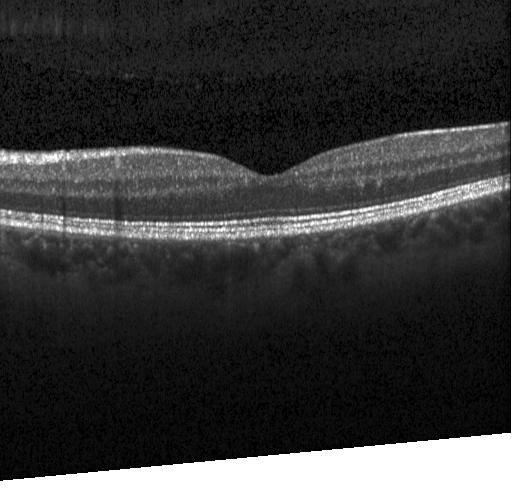
Optical coherence tomography scan. Through the macula — Impression: no choroidal neovascularization, diabetic macular edema, or drusen.